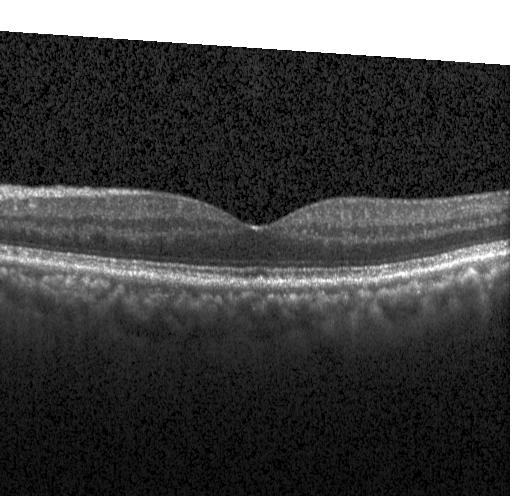
Impression: neither choroidal neovascularization, diabetic macular edema, nor drusen.